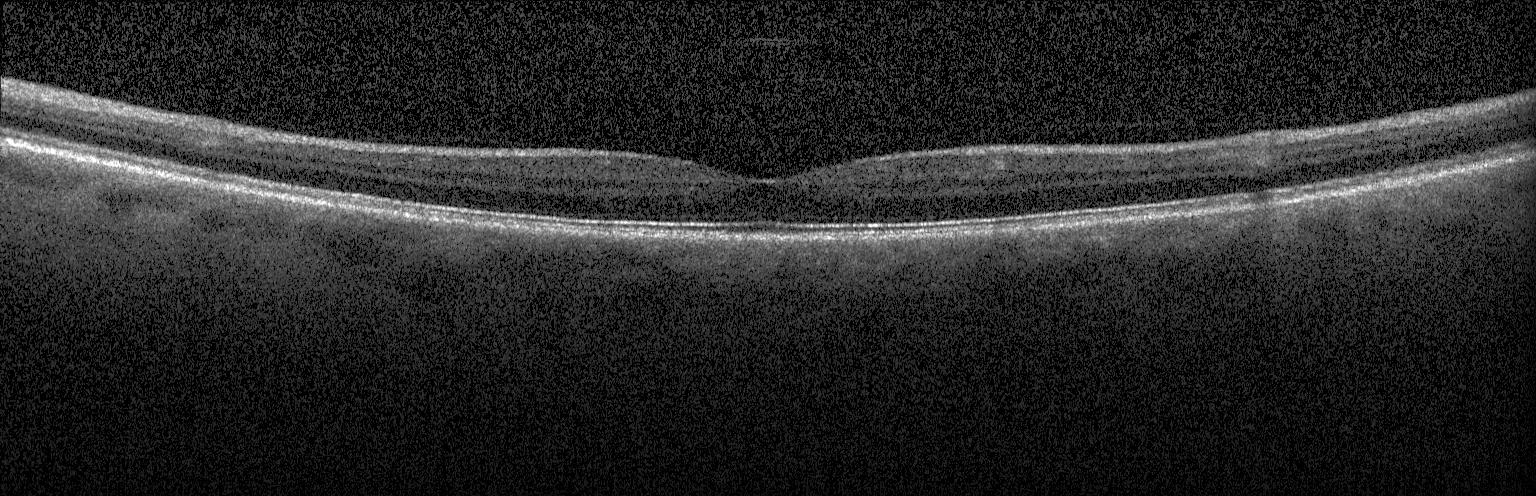
Macular OCT: no choroidal neovascularization, no diabetic macular edema, and no drusen.